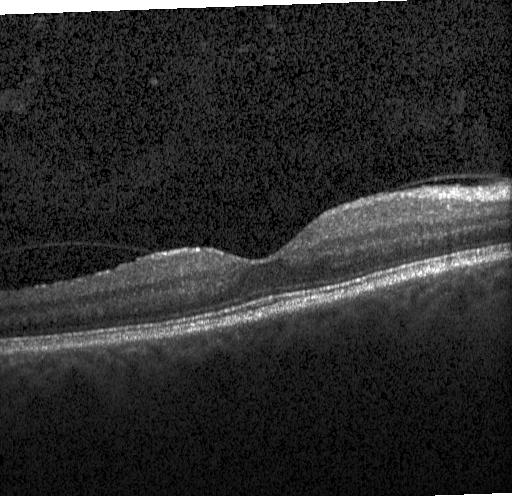
Impression: no choroidal neovascularization, no diabetic macular edema, and no drusen.